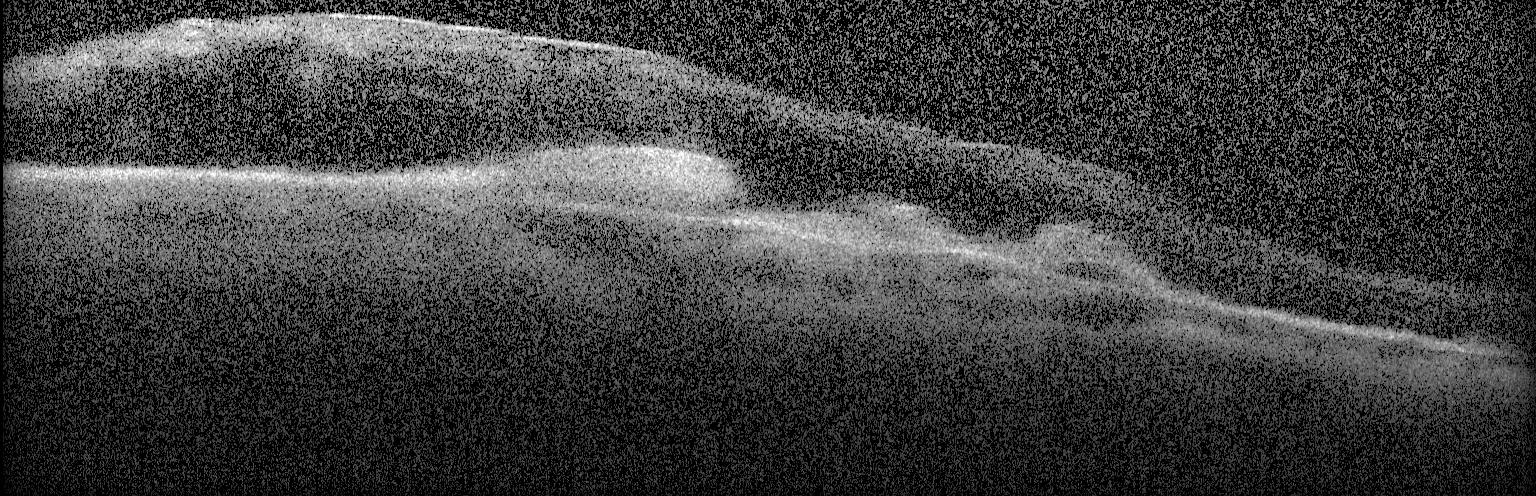

Heidelberg Spectralis, OCT line scan — Diagnosis: CNV.